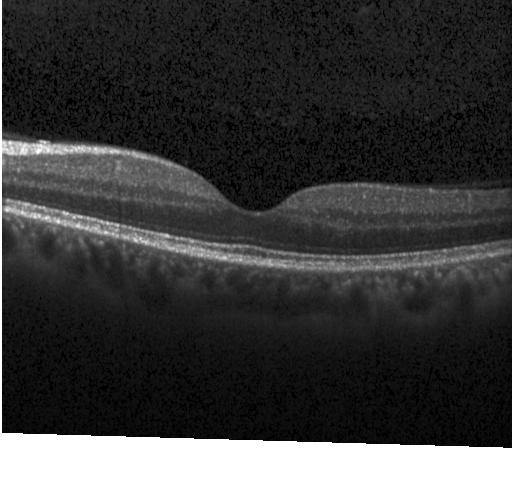

Through the macula, OCT line scan, spectral-domain OCT, Heidelberg Spectralis.
Dx: no choroidal neovascularization, diabetic macular edema, or drusen.